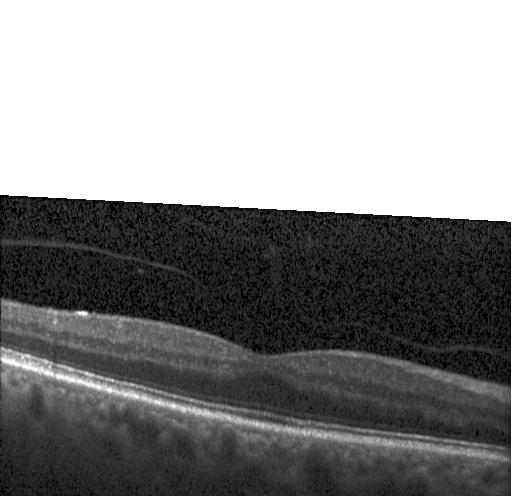
Impression: no choroidal neovascularization, diabetic macular edema, or drusen.